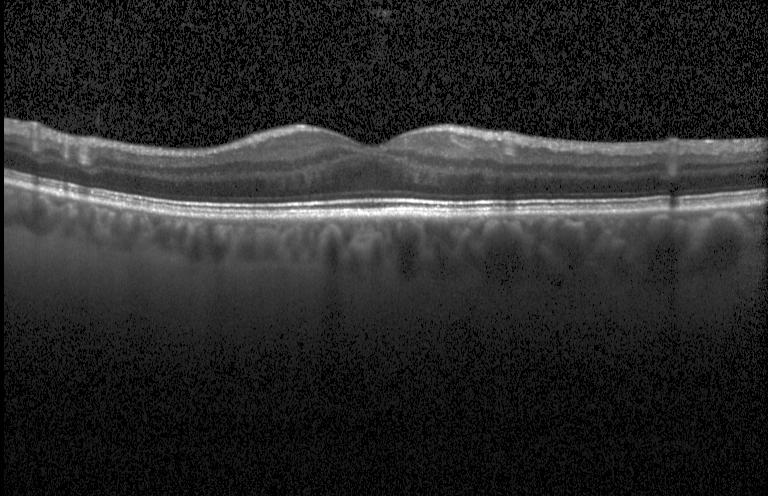
Macular OCT demonstrating no evidence of choroidal neovascularization, diabetic macular edema, or drusen.